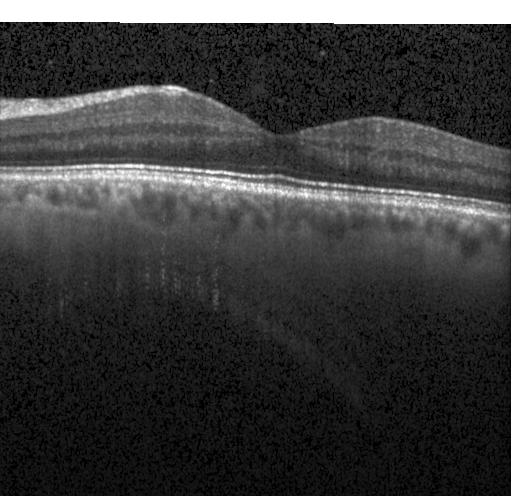 Retinal OCT B-scan, Heidelberg Spectralis OCT system, spectral-domain OCT — No choroidal neovascularization, diabetic macular edema, or drusen.